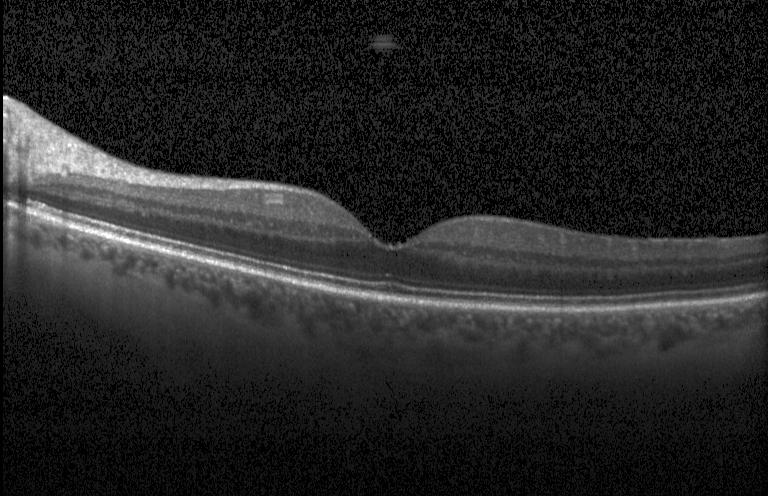
Macular OCT: no choroidal neovascularization, no diabetic macular edema, and no drusen.